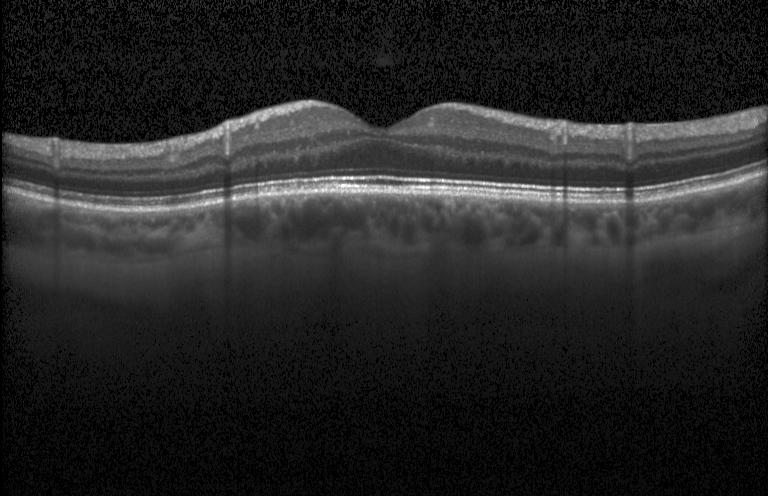
Optical coherence tomography scan — Diagnosis: no CNV, no DME, and no drusen.